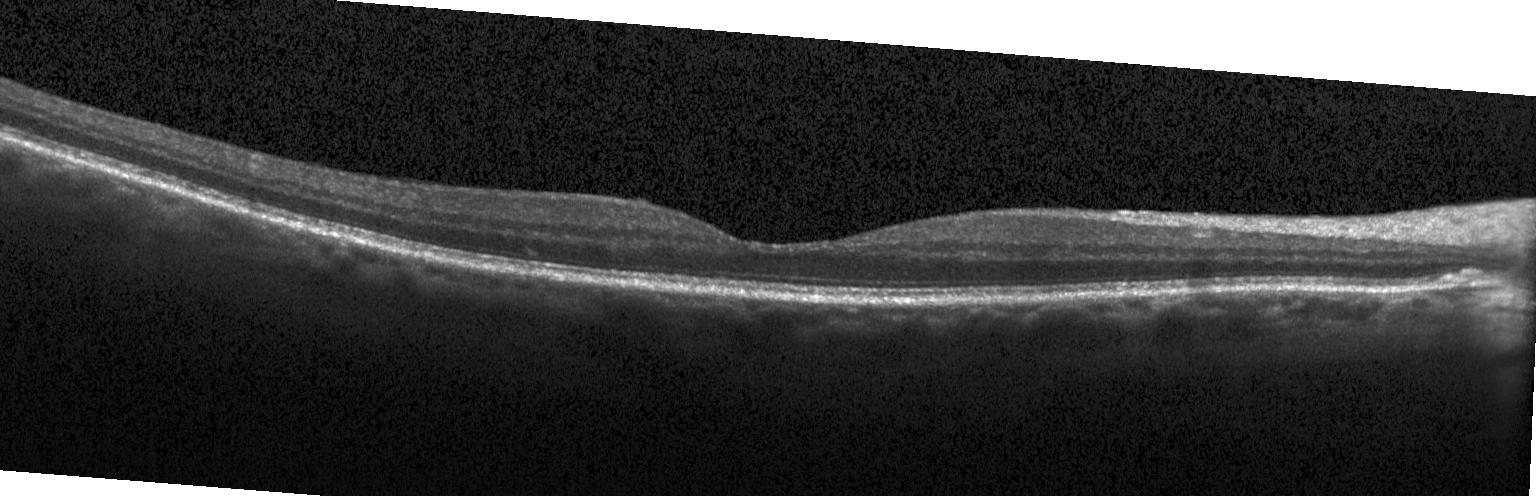
Optical coherence tomography B-scan.
No CNV, no DME, and no drusen.